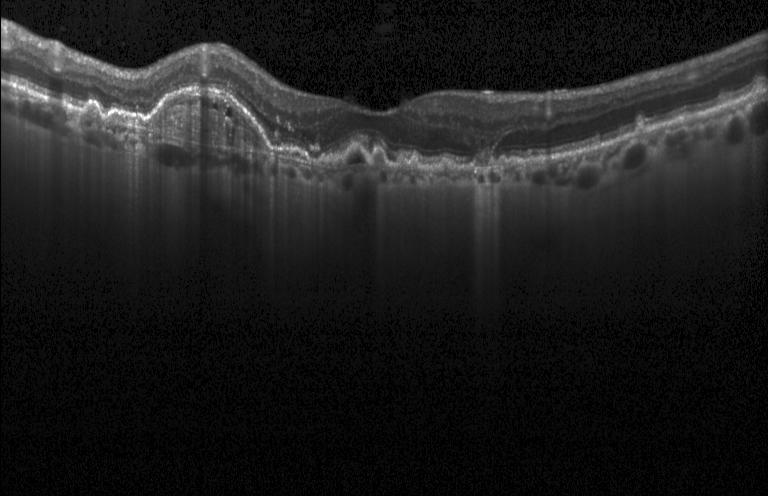

Impression: a choroidal neovascular membrane.